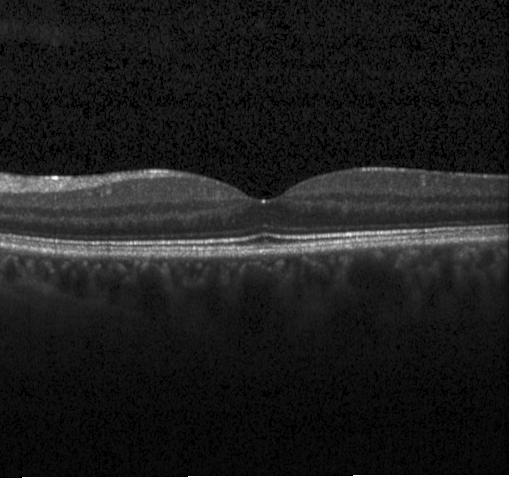 OCT line scan · SD-OCT · Heidelberg Spectralis. Diagnosis: no evidence of choroidal neovascularization, diabetic macular edema, or drusen.